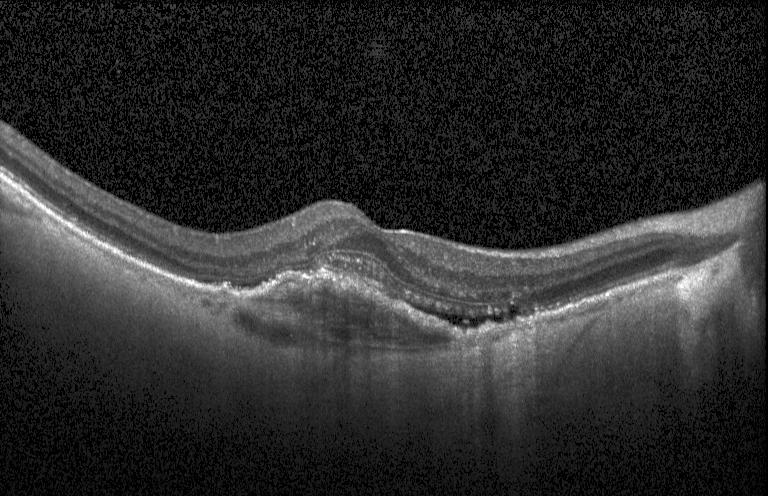

Horizontal scan through the fovea; retinal OCT B-scan.
Impression: a choroidal neovascular membrane.